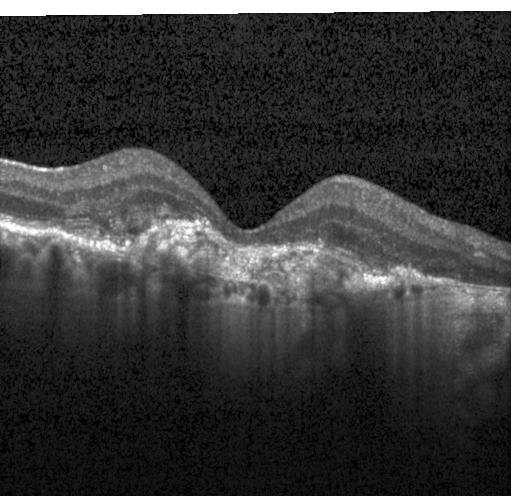

OCT B-scan
Assessment: a choroidal neovascular membrane.